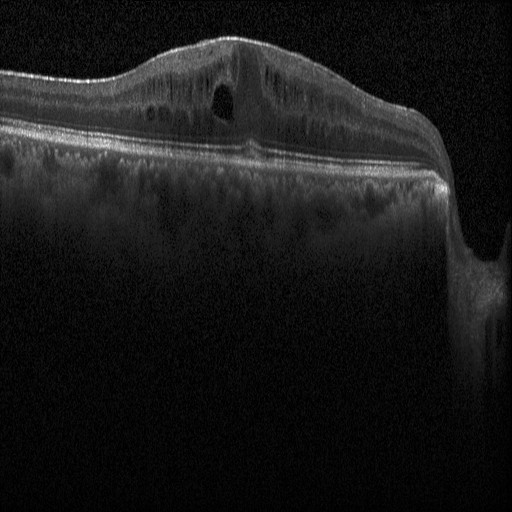

SD-OCT · horizontal scan through the fovea · retinal OCT B-scan · instrument: Heidelberg Spectralis — Assessment: diabetic macular edema (DME).